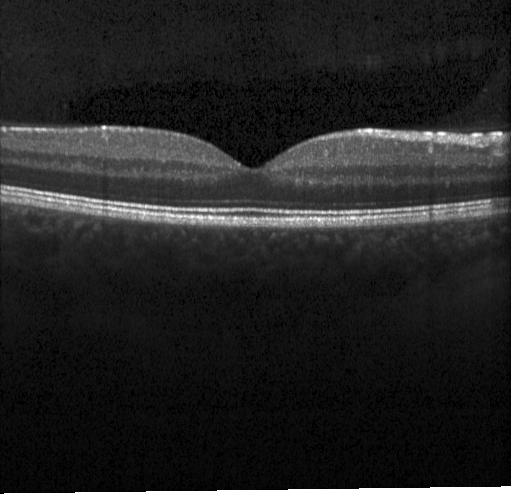 Macular OCT demonstrating neither CNV, DME, nor drusen.